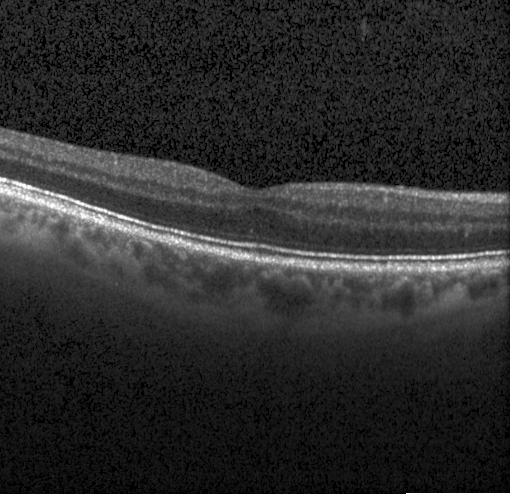

Centered on the fovea. Optical coherence tomography scan — Impression: no choroidal neovascularization, diabetic macular edema, or drusen.